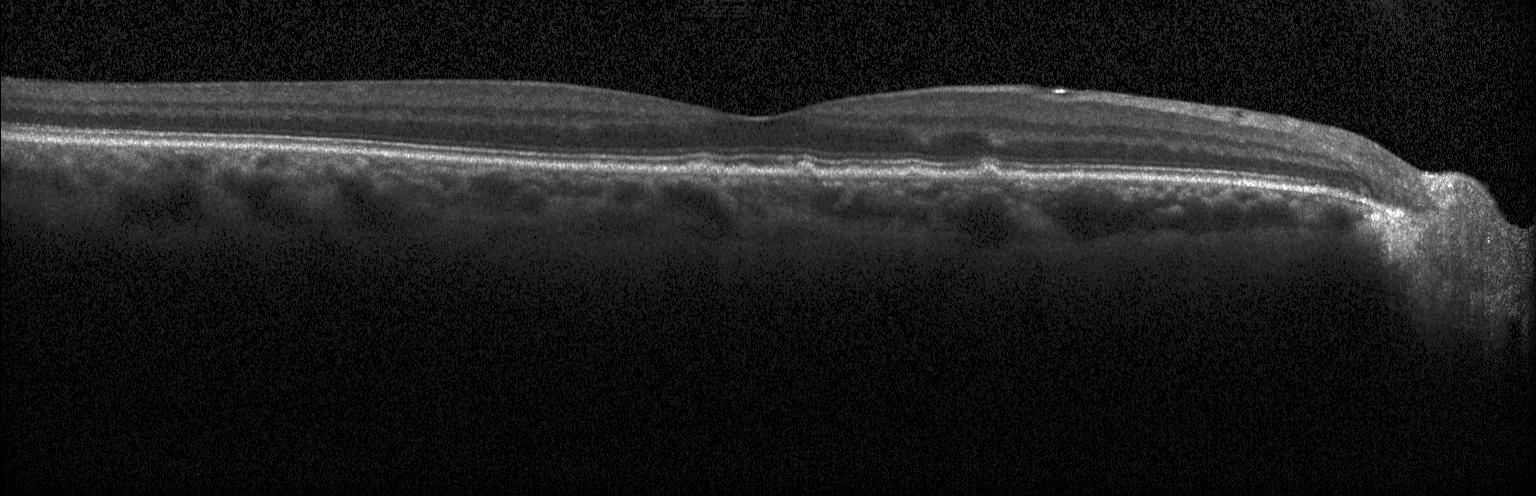
Acquired on a Heidelberg Spectralis. OCT line scan. SD-OCT. Centered on the fovea — Diagnosis: sub-RPE drusenoid deposits.